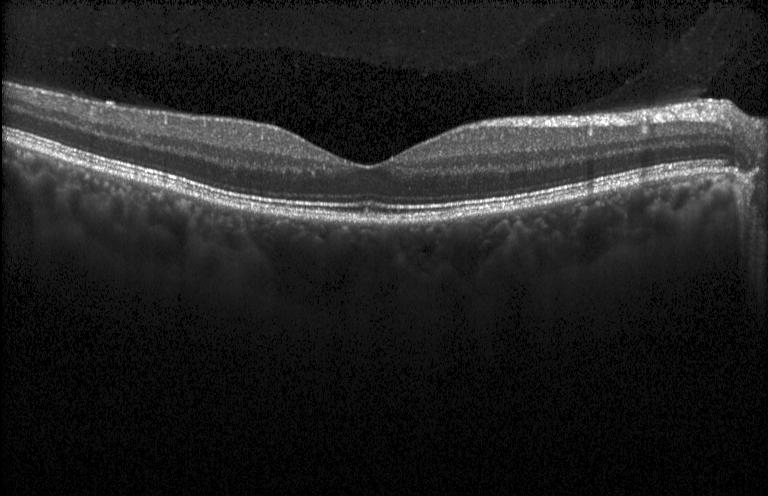

This B-scan demonstrates no choroidal neovascularization, no diabetic macular edema, and no drusen.